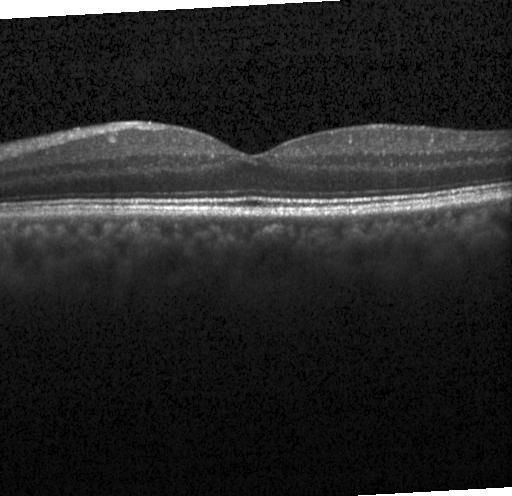
Horizontal scan through the fovea; retinal OCT cross-section; SD-OCT; acquired on a Heidelberg Spectralis. Finding: no evidence of choroidal neovascularization, diabetic macular edema, or drusen.